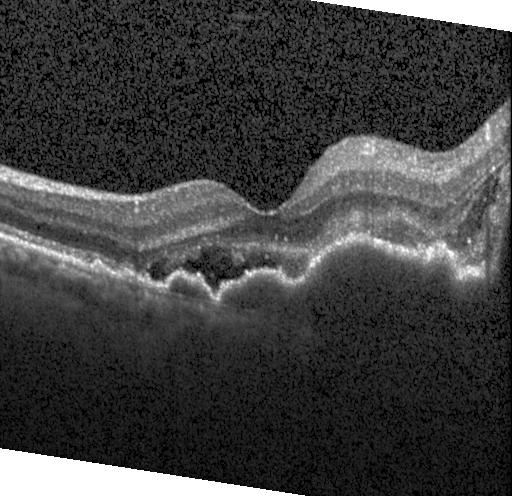 Heidelberg Spectralis, SD-OCT, fovea-centered, optical coherence tomography B-scan. Impression: choroidal neovascularization.